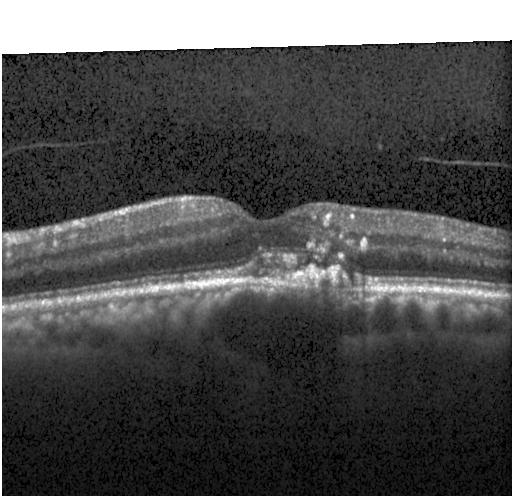

Spectral-domain OCT. OCT line scan.
Diagnosis: a choroidal neovascular membrane.